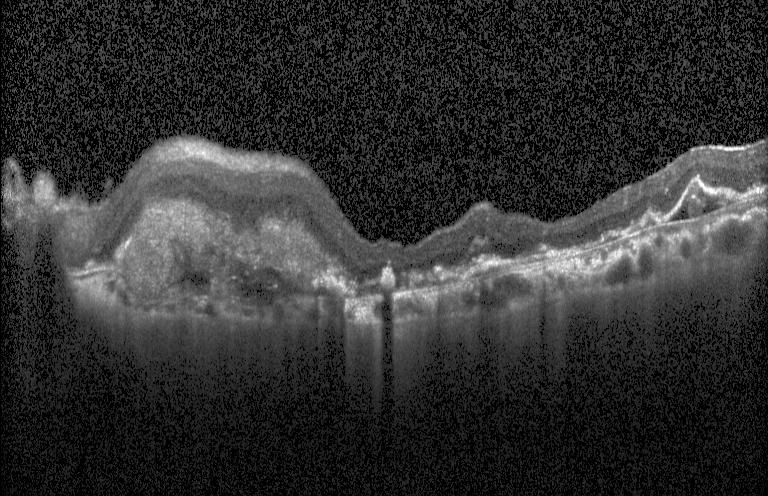
Diagnosis: CNV.